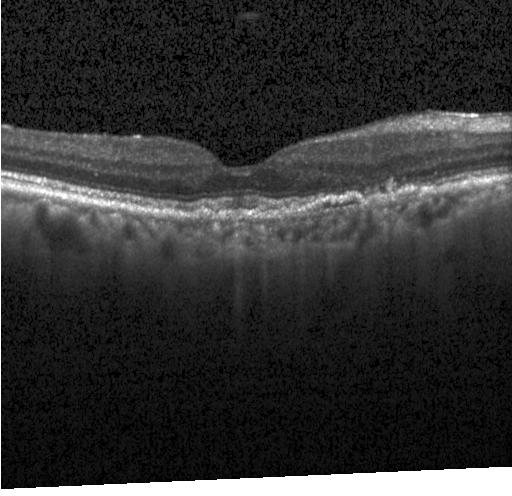 Spectral-domain optical coherence tomography; optical coherence tomography scan
A choroidal neovascular membrane.